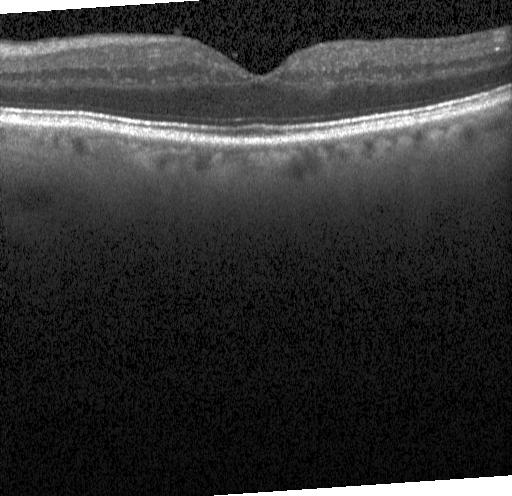 Retinal OCT cross-section. SD-OCT.
No evidence of CNV, DME, or drusen.